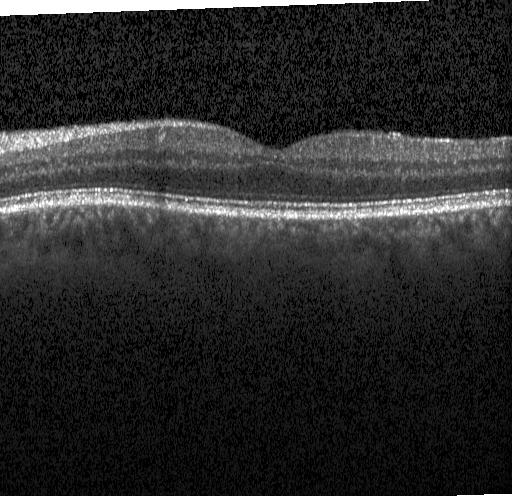 Impression: no choroidal neovascularization, no diabetic macular edema, and no drusen.